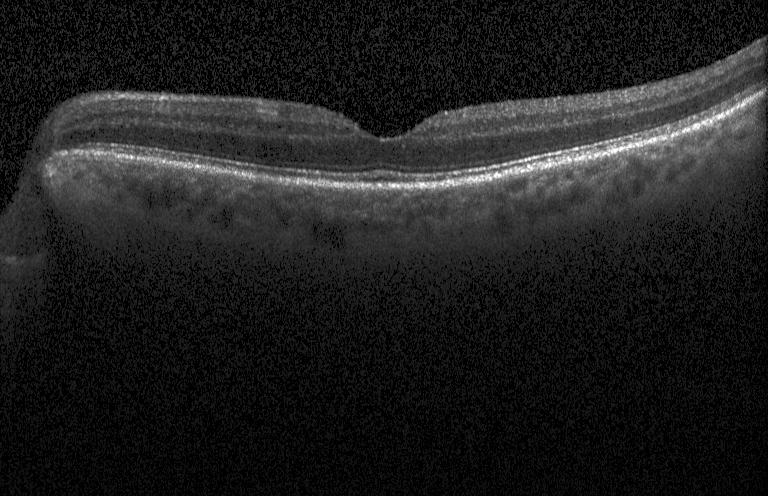
Retinal OCT cross-section — The scan shows neither choroidal neovascularization, diabetic macular edema, nor drusen.